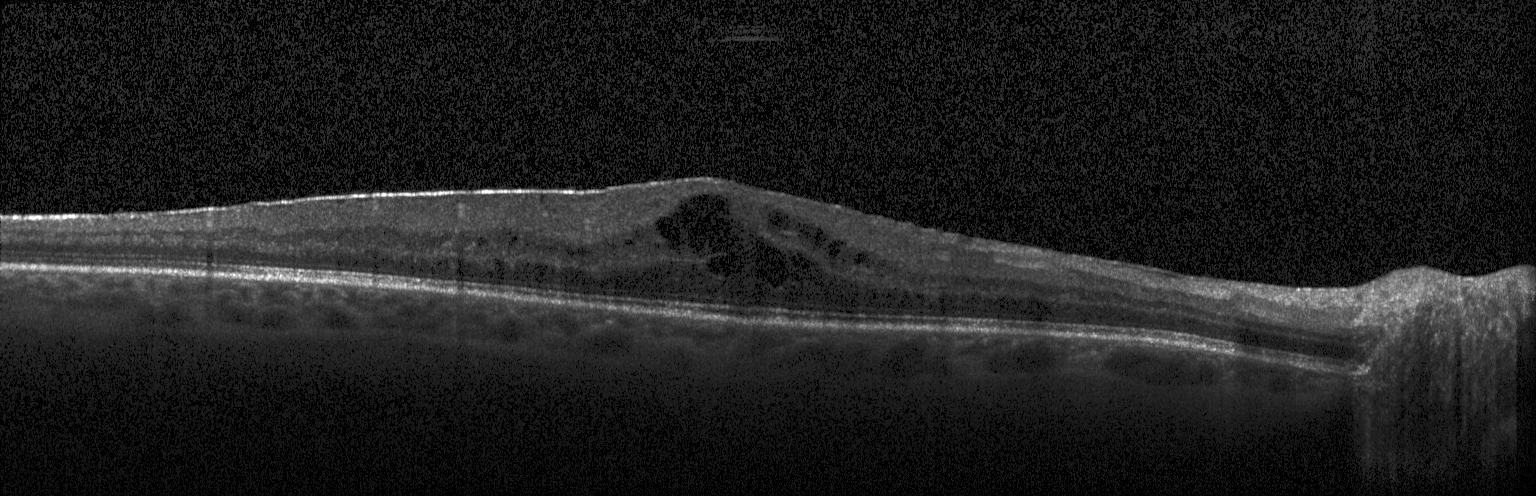

Spectral-domain OCT B-scan: diabetic macular edema (DME).